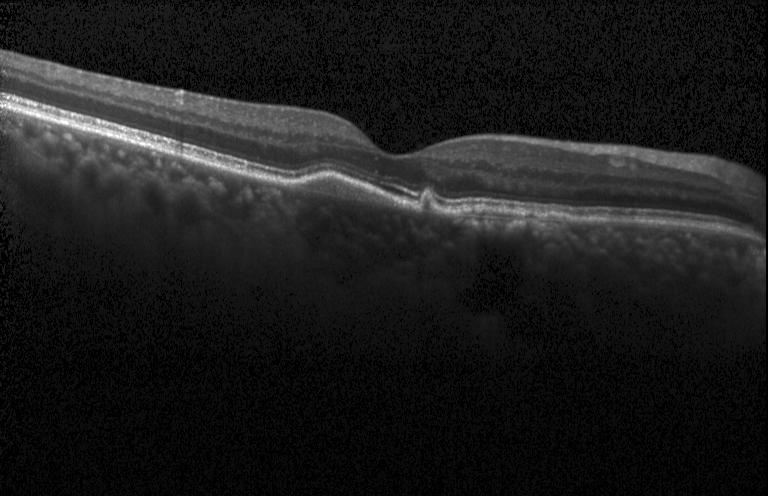

OCT line scan.
This B-scan demonstrates multiple drusen.